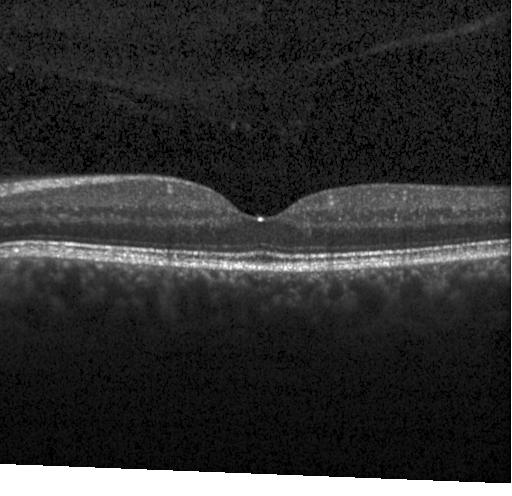 Dx: no choroidal neovascularization, diabetic macular edema, or drusen.